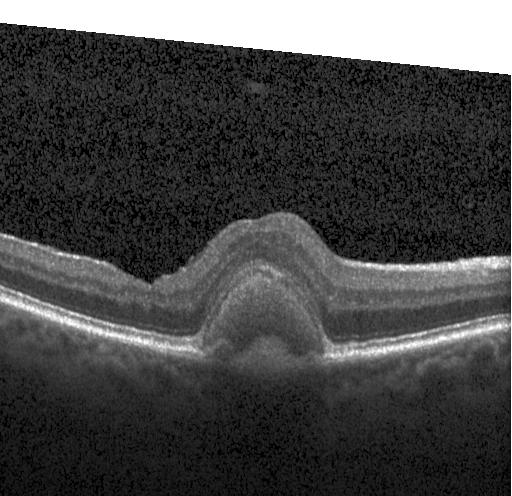 Retinal OCT cross-section · spectral-domain OCT · centered on the fovea — Assessment: a choroidal neovascular membrane.